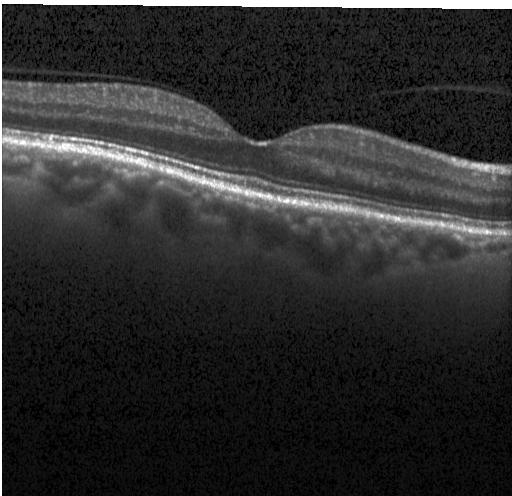
Assessment: no evidence of choroidal neovascularization, diabetic macular edema, or drusen.